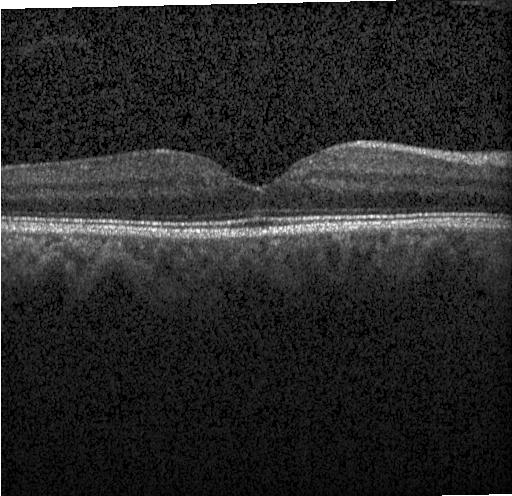 OCT finding: no choroidal neovascularization, diabetic macular edema, or drusen.